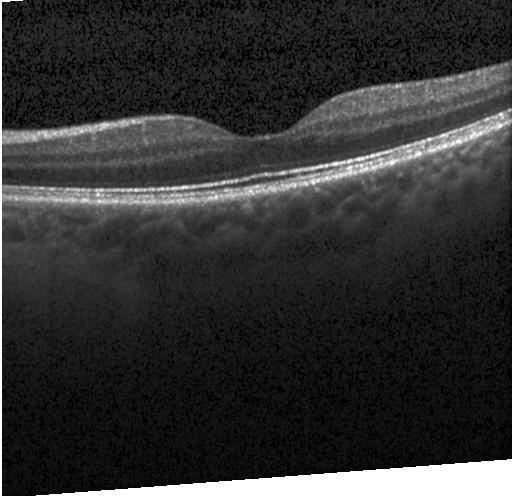 Diagnosis: no evidence of CNV, DME, or drusen.